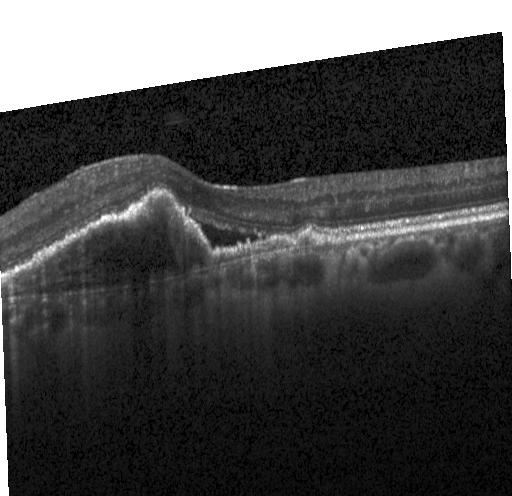 Retinal OCT B-scan · Heidelberg Spectralis — The scan shows choroidal neovascularization (CNV).